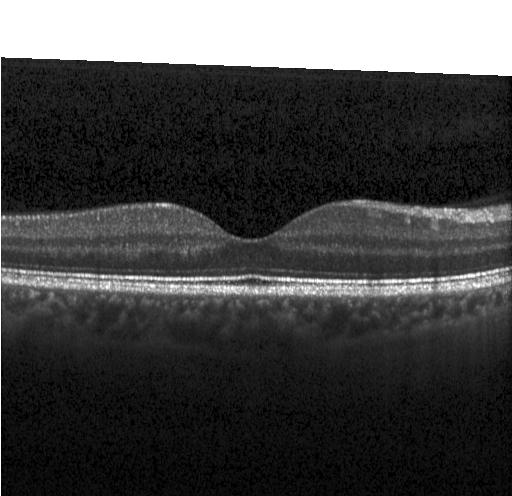
Retinal OCT cross-section; acquired on a Heidelberg Spectralis
Finding: no evidence of CNV, DME, or drusen.